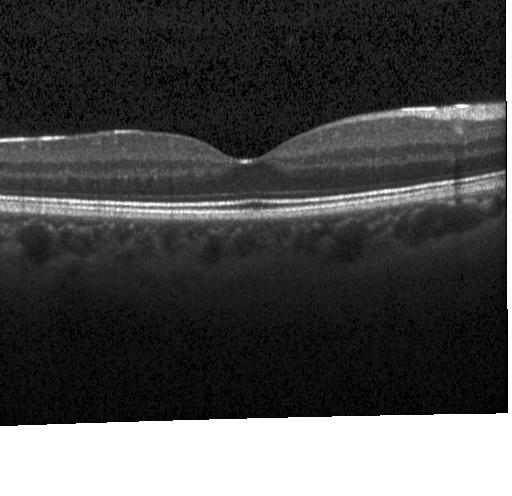
Macular OCT: no evidence of CNV, DME, or drusen.